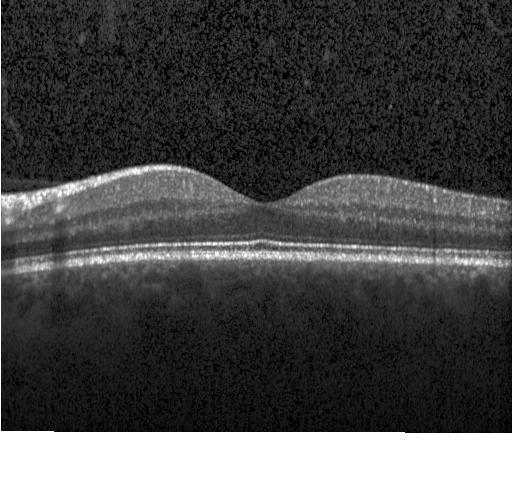 Spectral-domain OCT · optical coherence tomography B-scan · instrument: Heidelberg Spectralis. Assessment: no evidence of CNV, DME, or drusen.